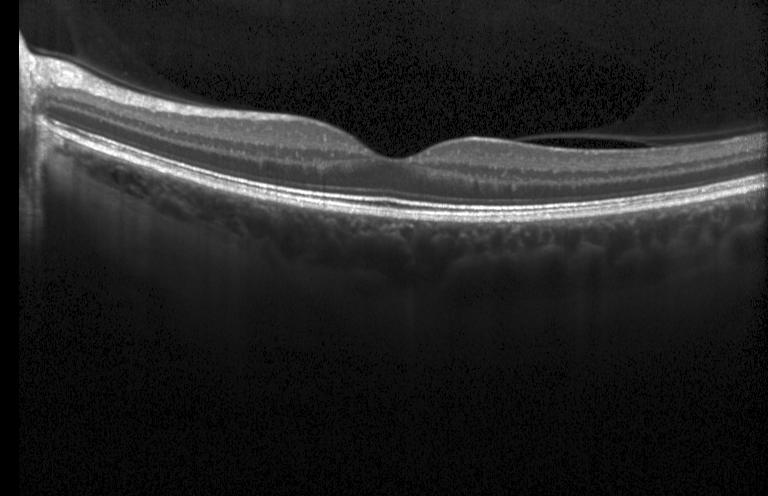

OCT line scan. Neither choroidal neovascularization, diabetic macular edema, nor drusen.